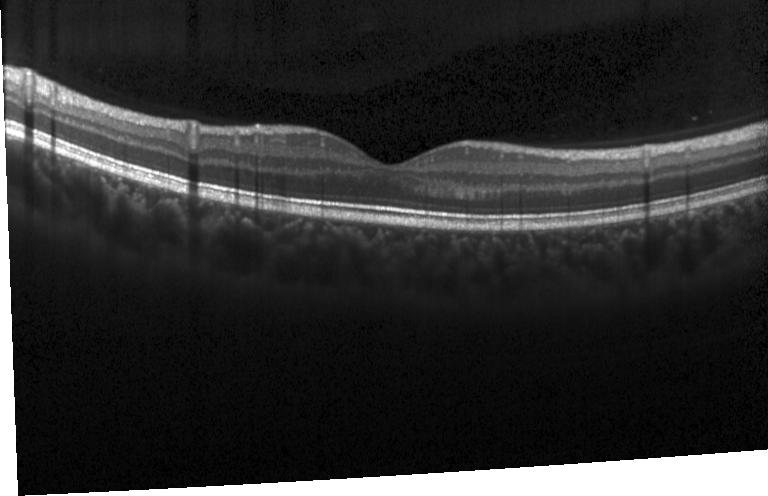
Retinal OCT B-scan · Heidelberg Spectralis OCT system · horizontal scan through the fovea · SD-OCT.
No evidence of choroidal neovascularization, diabetic macular edema, or drusen.